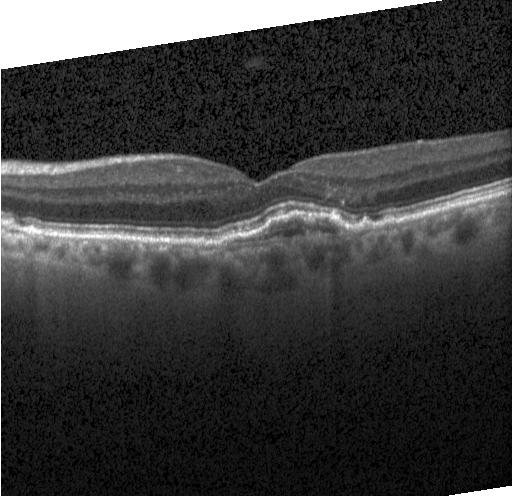
Through the macula · optical coherence tomography scan
Finding: choroidal neovascularization.